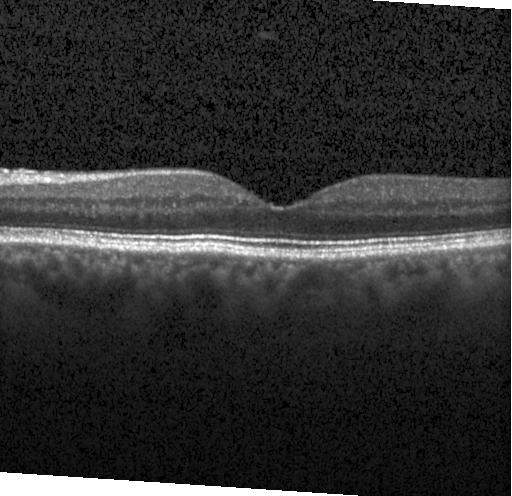

OCT finding: no evidence of choroidal neovascularization, diabetic macular edema, or drusen.